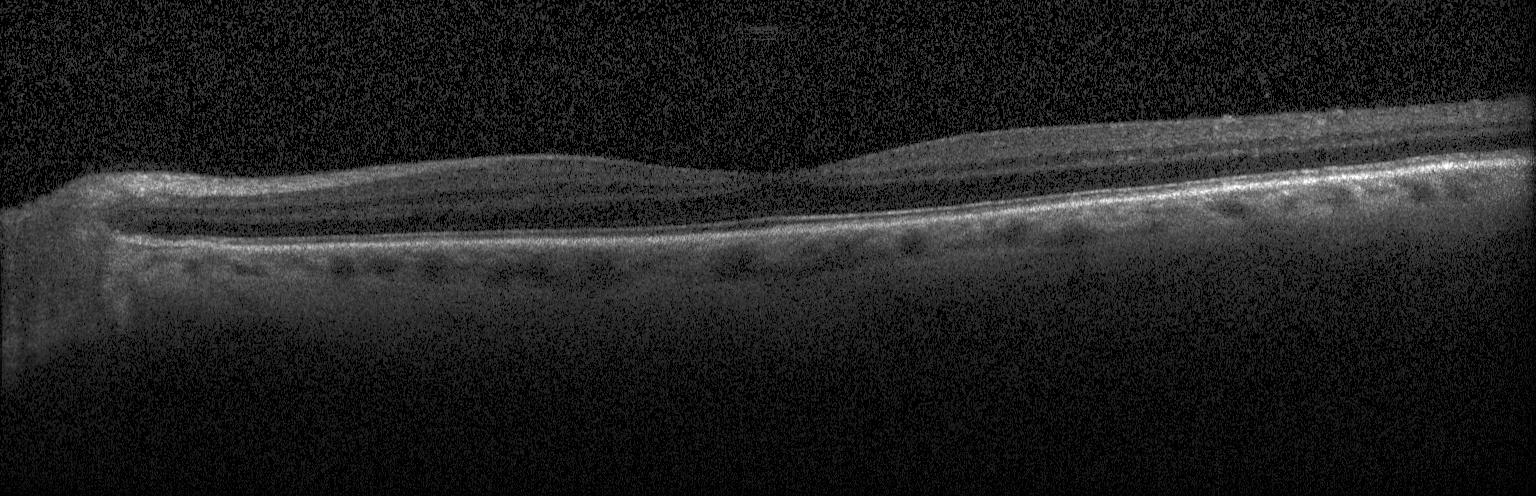
OCT B-scan showing neither CNV, DME, nor drusen.